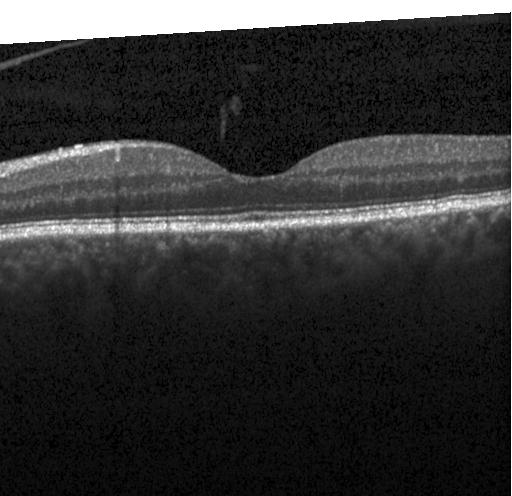 OCT line scan.
No CNV, no DME, and no drusen.